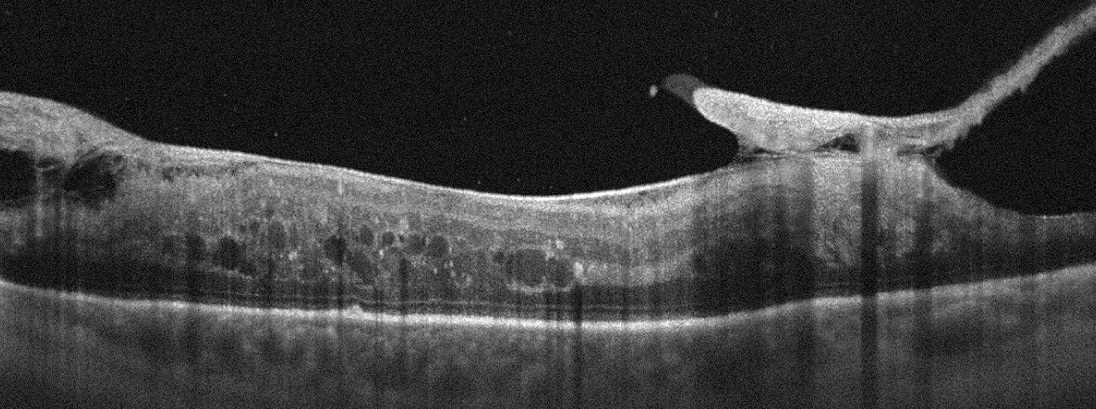 Finding: diabetic macular edema.